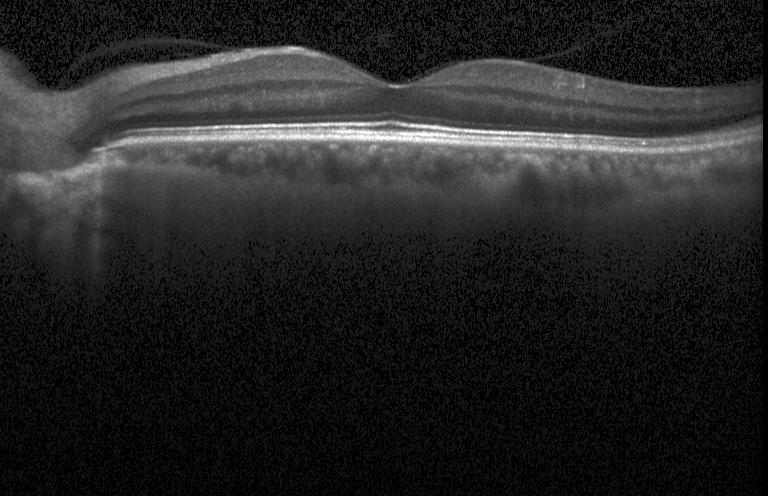

Spectral-domain optical coherence tomography · centered on the fovea · optical coherence tomography B-scan · Heidelberg Spectralis.
Neither choroidal neovascularization, diabetic macular edema, nor drusen.